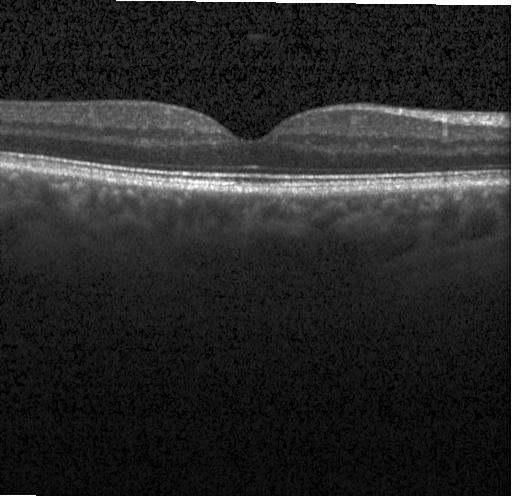

Instrument: Heidelberg Spectralis · OCT line scan · macular scan.
This B-scan demonstrates no choroidal neovascularization, diabetic macular edema, or drusen.